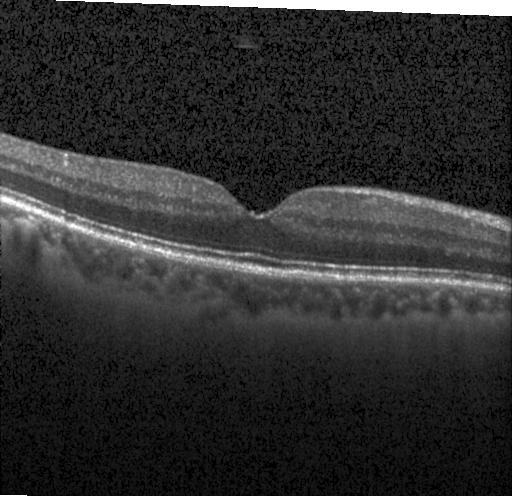 Spectral-domain OCT; OCT B-scan. Finding: neither choroidal neovascularization, diabetic macular edema, nor drusen.